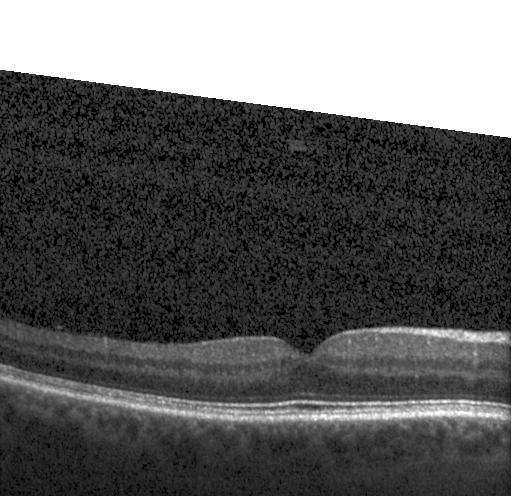
OCT B-scan. Centered on the fovea. Spectral-domain OCT — Diagnosis: no choroidal neovascularization, no diabetic macular edema, and no drusen.